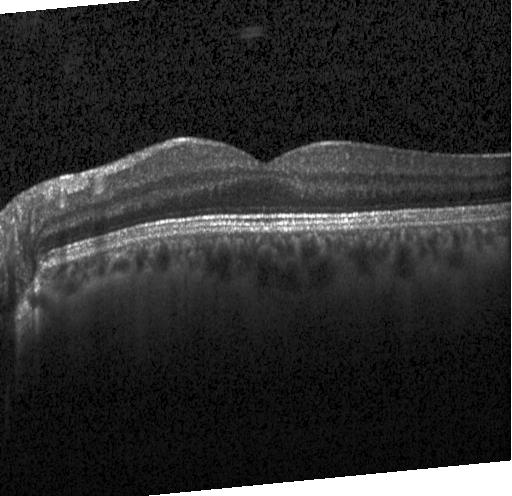
Finding: no evidence of choroidal neovascularization, diabetic macular edema, or drusen.